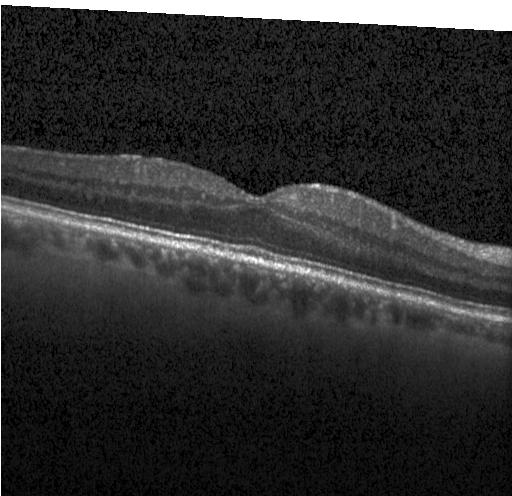 Finding: no choroidal neovascularization, diabetic macular edema, or drusen.